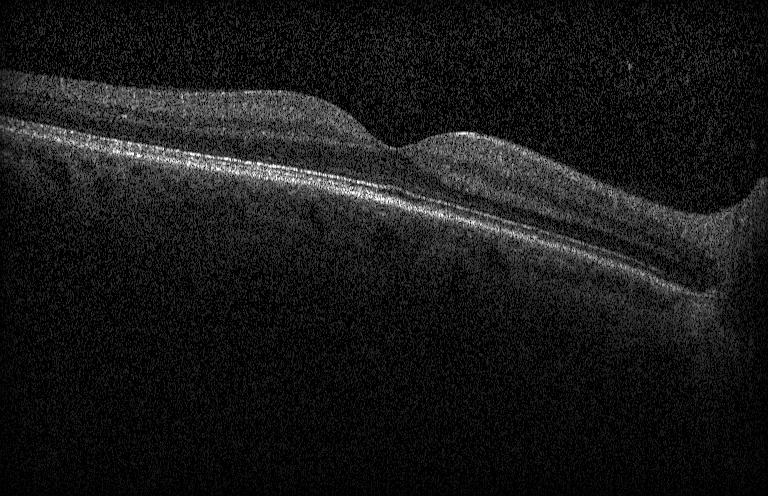

Diagnosis: no evidence of choroidal neovascularization, diabetic macular edema, or drusen.